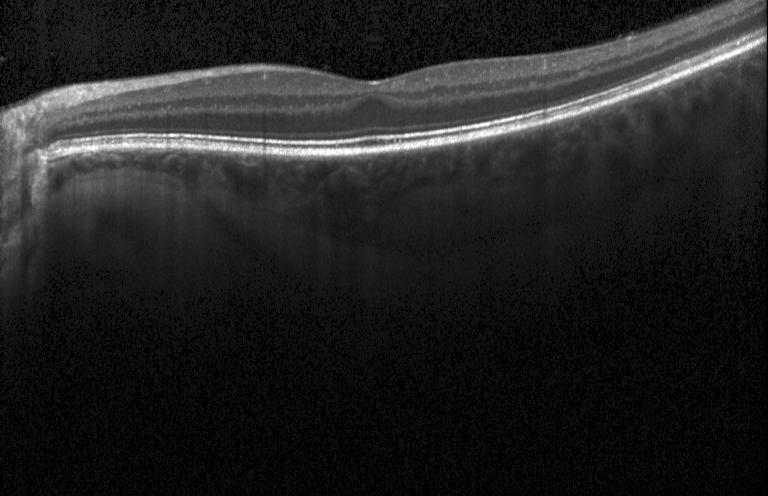

Fovea-centered. Acquired on a Heidelberg Spectralis. Spectral-domain OCT. Optical coherence tomography B-scan. Macular OCT: no CNV, no DME, and no drusen.